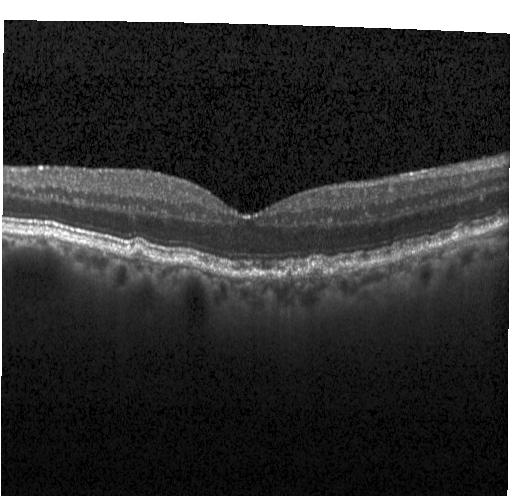
Sub-RPE drusenoid deposits.